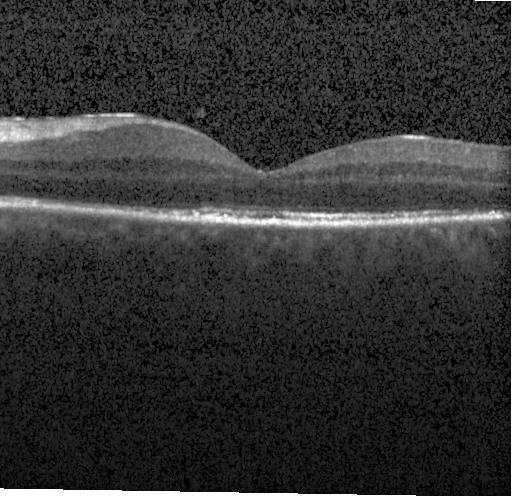

The scan shows no choroidal neovascularization, diabetic macular edema, or drusen.